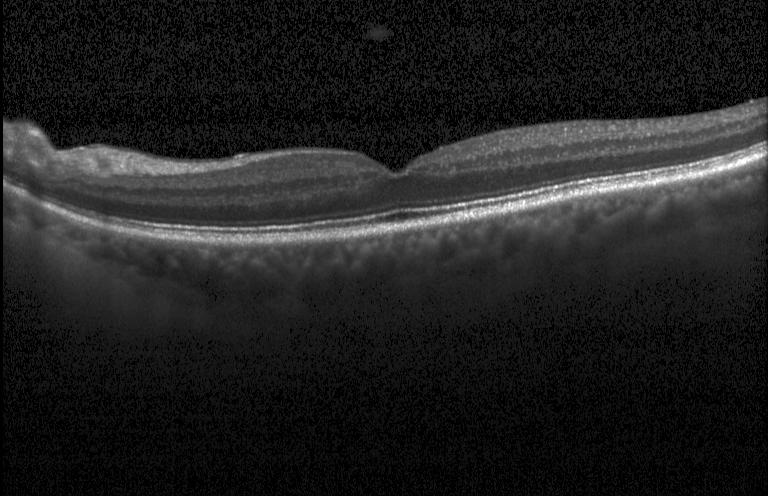

Optical coherence tomography scan — Finding: no CNV, no DME, and no drusen.